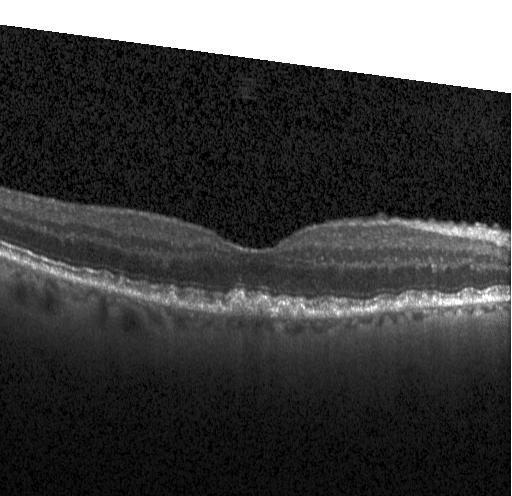

Centered on the fovea, optical coherence tomography B-scan, Heidelberg Spectralis OCT system.
The scan shows sub-RPE drusenoid deposits.